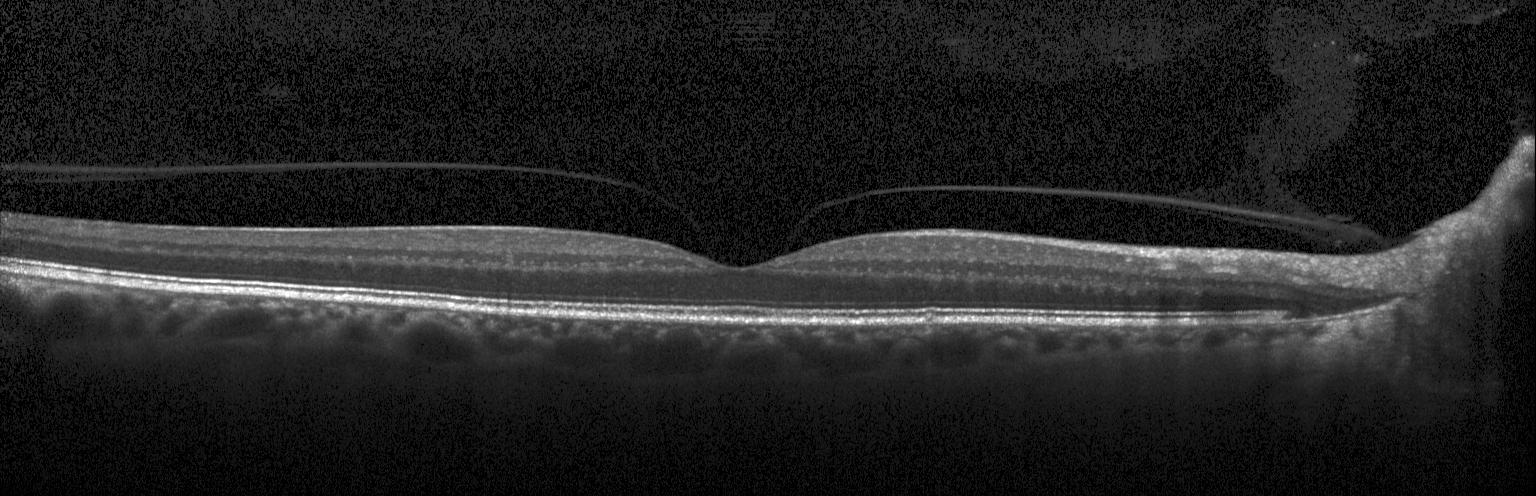
Diagnosis: no choroidal neovascularization, diabetic macular edema, or drusen.